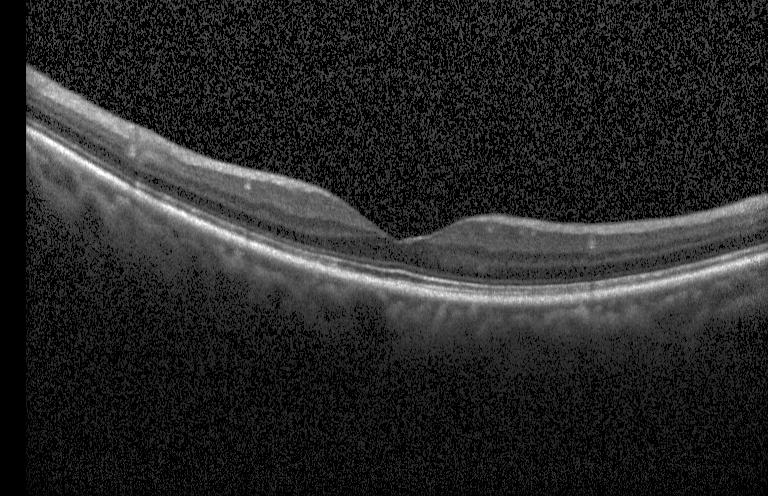 Centered on the fovea; acquired on a Heidelberg Spectralis; spectral-domain optical coherence tomography; optical coherence tomography B-scan.
Assessment: no evidence of choroidal neovascularization, diabetic macular edema, or drusen.